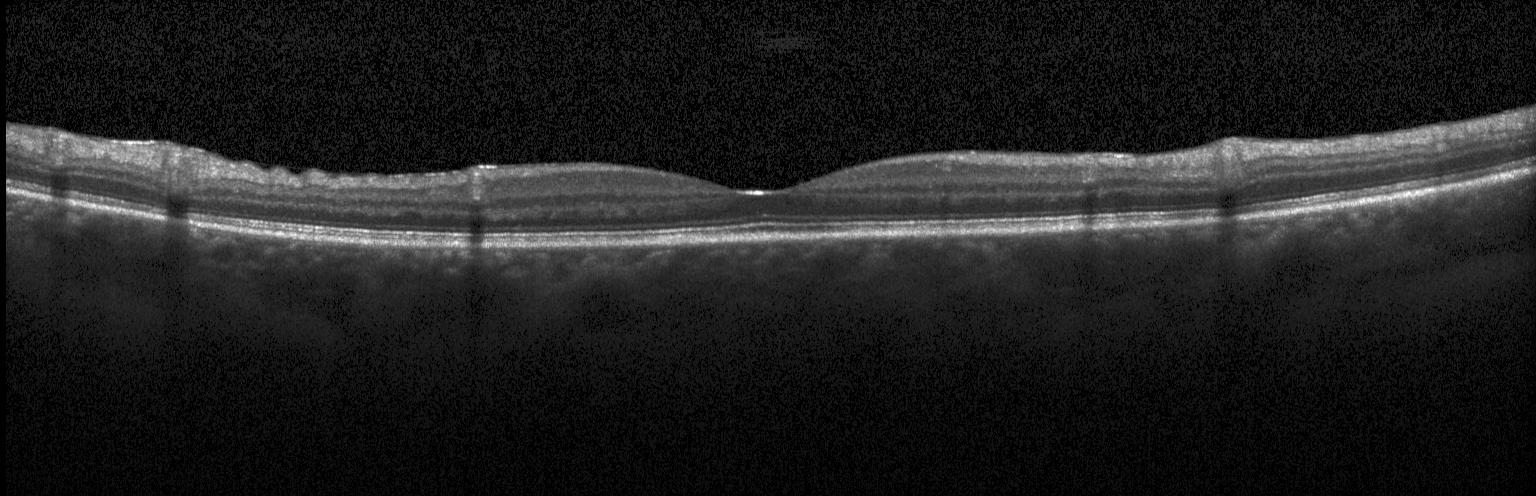

Optical coherence tomography B-scan.
This B-scan demonstrates neither CNV, DME, nor drusen.